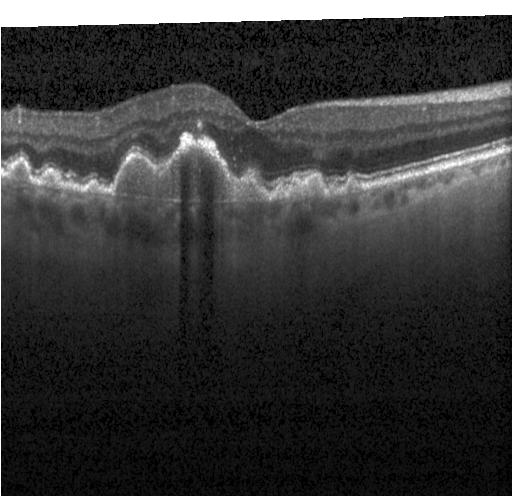 Spectral-domain OCT B-scan: choroidal neovascularization.